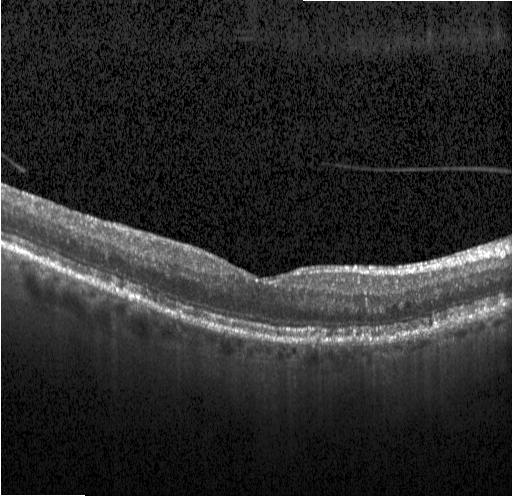 Optical coherence tomography scan. The scan shows multiple drusen.